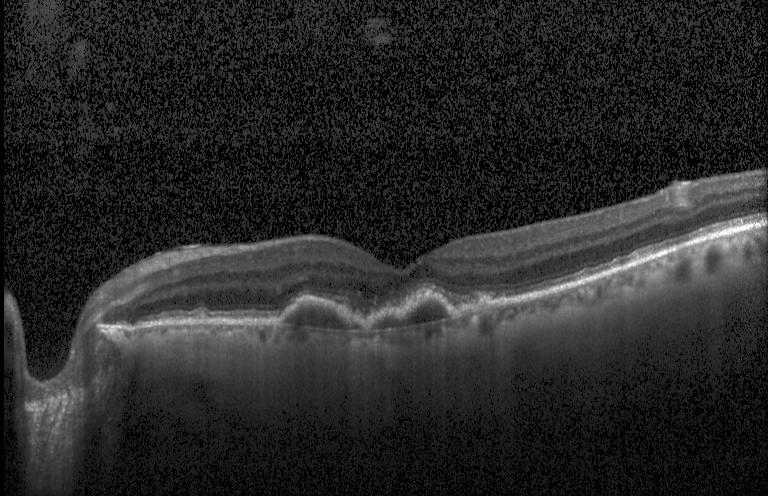

Through the macula. Acquired on a Heidelberg Spectralis. Optical coherence tomography B-scan. Spectral-domain optical coherence tomography.
Macular OCT: a choroidal neovascular membrane.